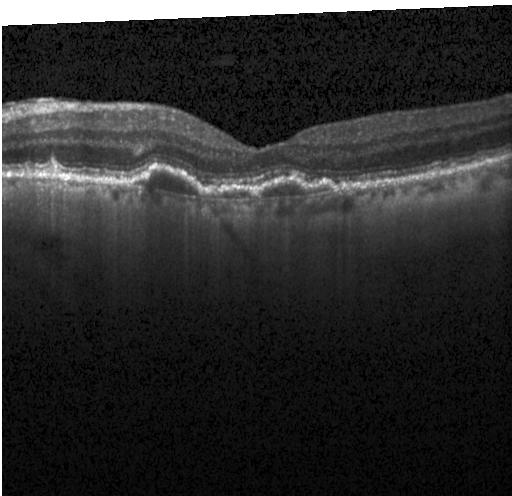 OCT B-scan showing choroidal neovascularization (CNV).